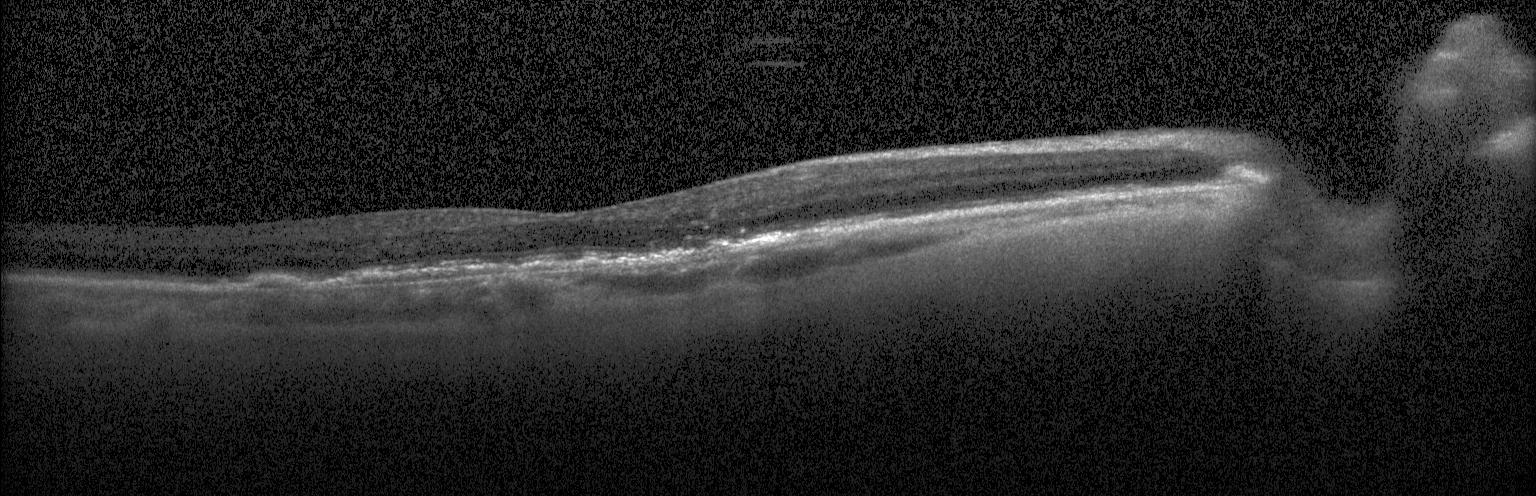

Fovea-centered. Optical coherence tomography B-scan. Acquired on a Heidelberg Spectralis
Diagnosis: a choroidal neovascular membrane.